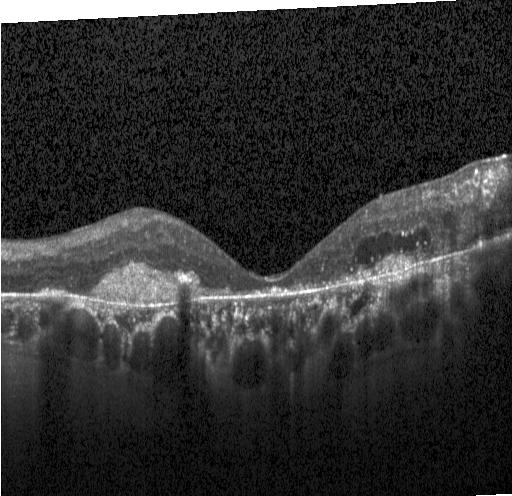
Optical coherence tomography scan, centered on the fovea, SD-OCT.
Diagnosis: CNV.